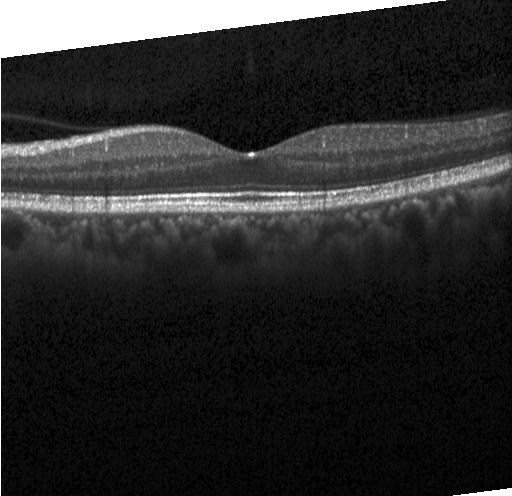

OCT B-scan. Horizontal scan through the fovea. SD-OCT — Diagnosis: no CNV, no DME, and no drusen.